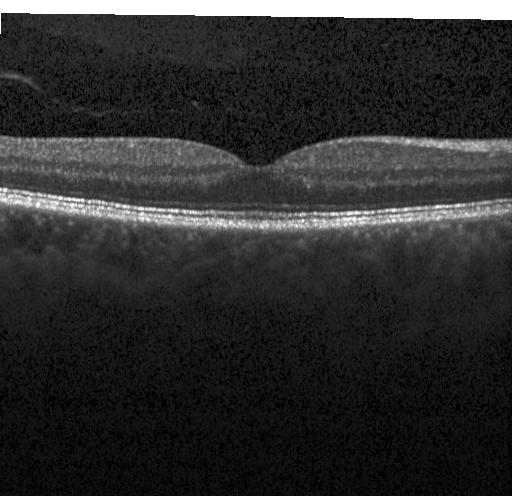

OCT B-scan; Heidelberg Spectralis.
The scan shows no choroidal neovascularization, no diabetic macular edema, and no drusen.